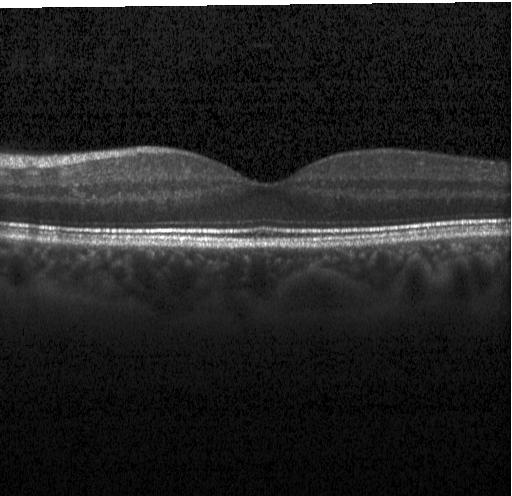
Optical coherence tomography B-scan. Macular OCT: no choroidal neovascularization, no diabetic macular edema, and no drusen.